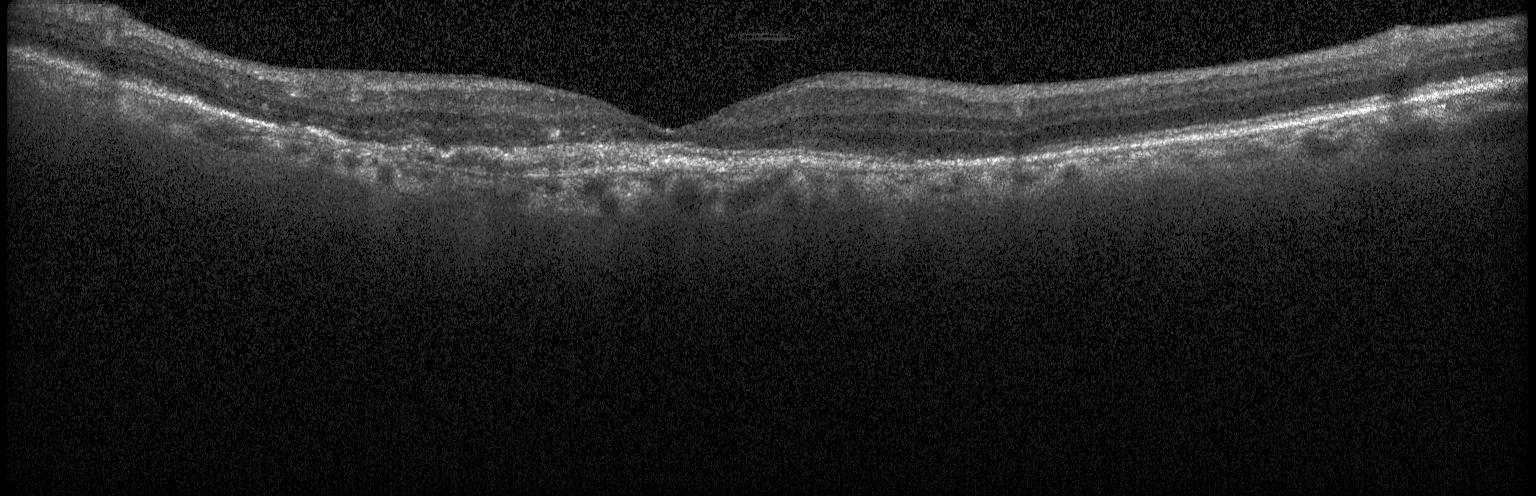
The scan shows a choroidal neovascular membrane.